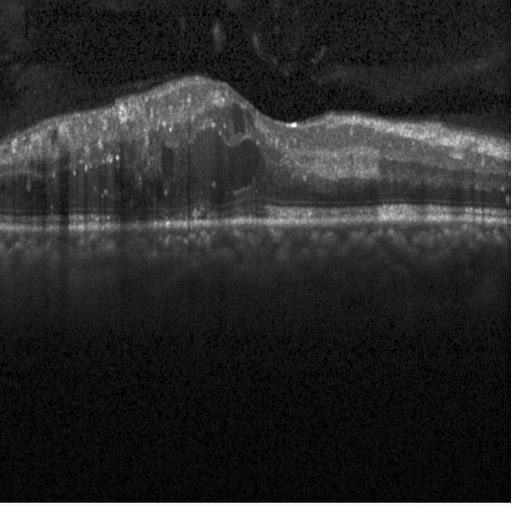

OCT line scan. Acquired on a Heidelberg Spectralis.
Finding: DME.